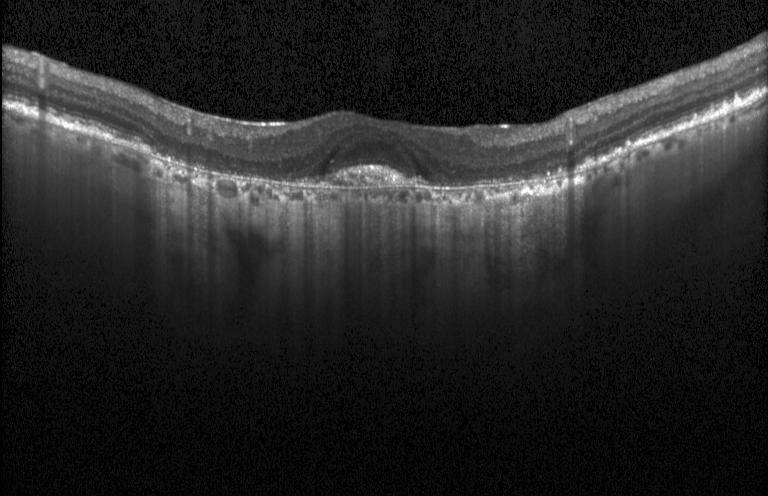

Diagnosis: CNV.